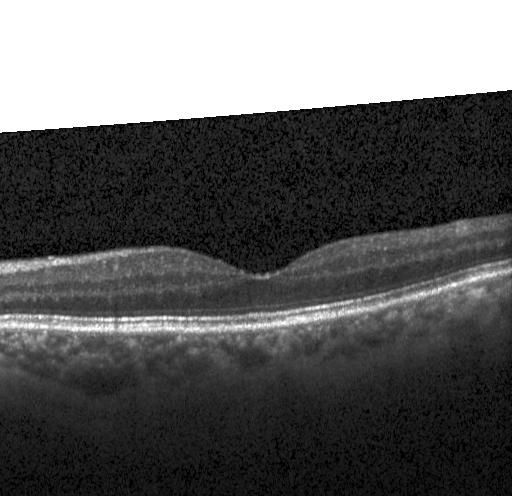 OCT scan showing neither choroidal neovascularization, diabetic macular edema, nor drusen.